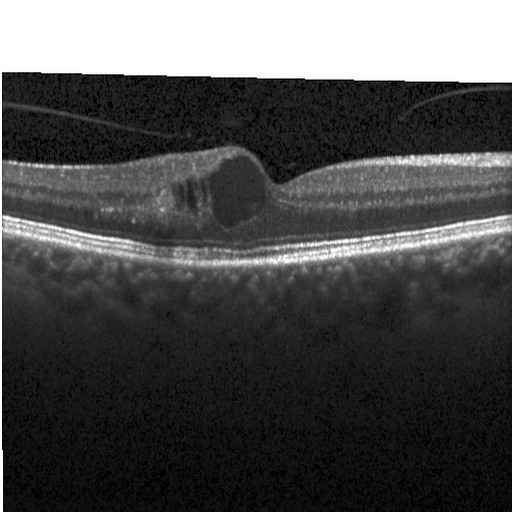

Macular OCT: DME.